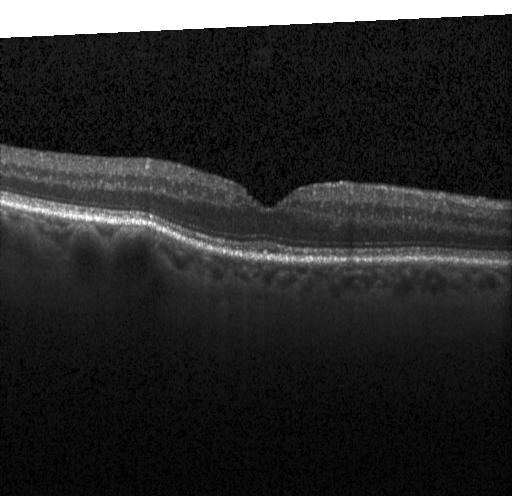
OCT B-scan showing no choroidal neovascularization, diabetic macular edema, or drusen.